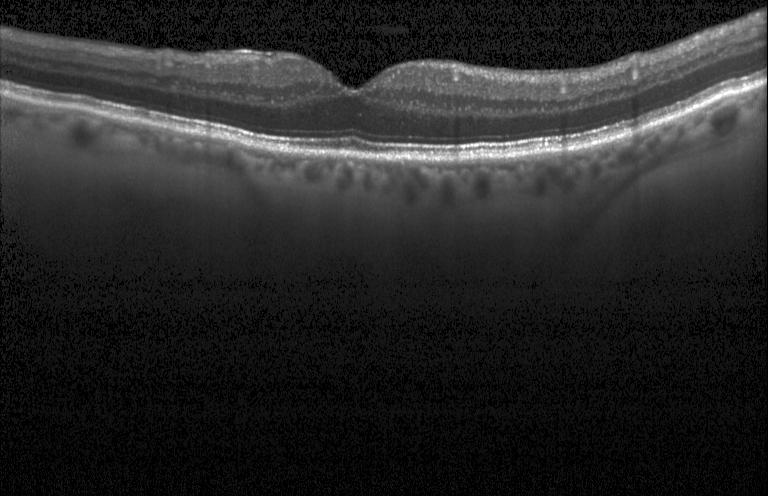
Spectral-domain OCT, OCT line scan
No CNV, no DME, and no drusen.